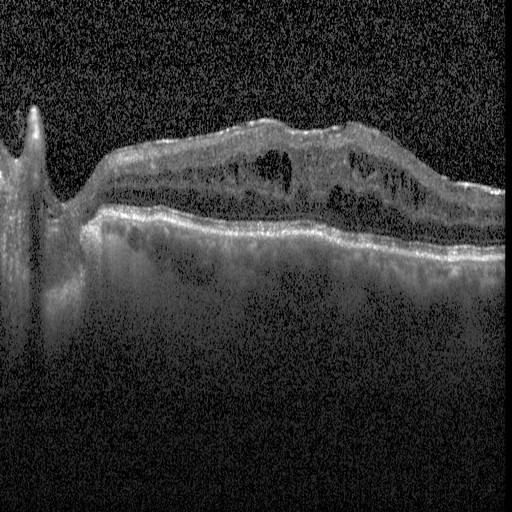
Finding: diabetic macular edema (DME).